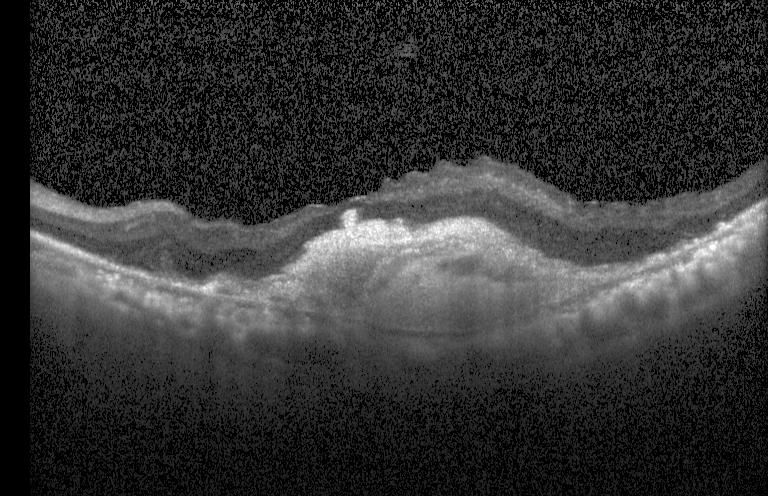 Spectral-domain OCT B-scan: choroidal neovascularization.